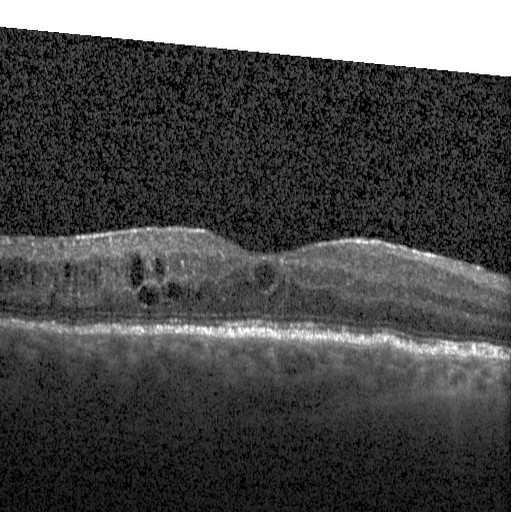 Retinal OCT cross-section showing diabetic macular edema (DME).